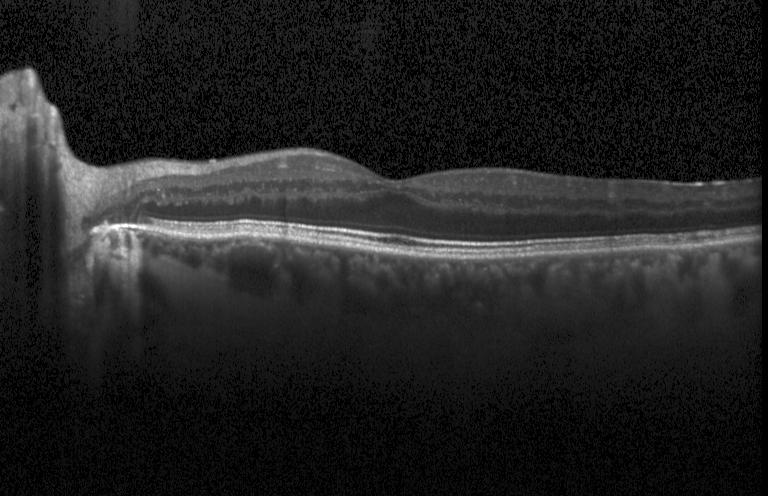 OCT line scan · Heidelberg Spectralis OCT system
This B-scan demonstrates no choroidal neovascularization, no diabetic macular edema, and no drusen.